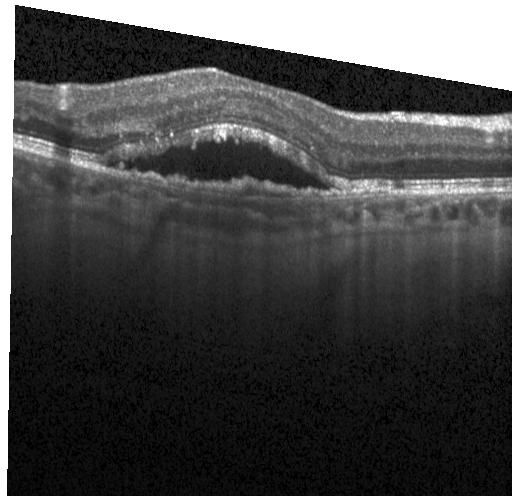

OCT line scan · instrument: Heidelberg Spectralis.
Diagnosis: a choroidal neovascular membrane.